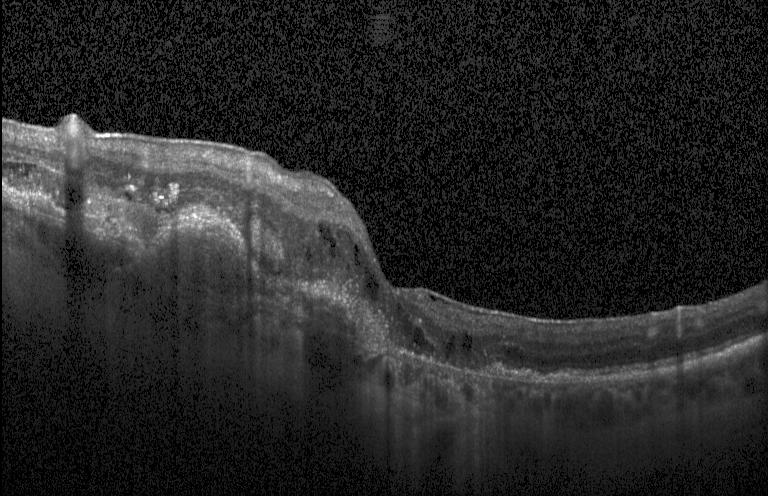
Retinal OCT B-scan; acquired on a Heidelberg Spectralis
Diagnosis: choroidal neovascularization (CNV).